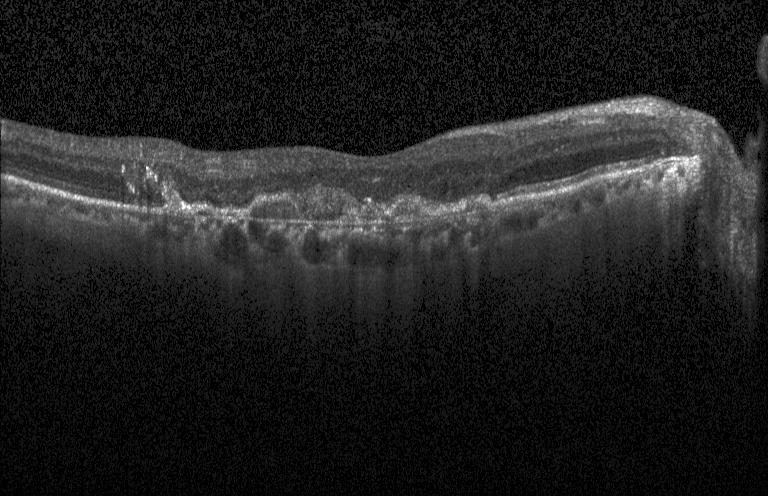 Through the macula, retinal OCT B-scan. OCT finding: choroidal neovascularization (CNV).